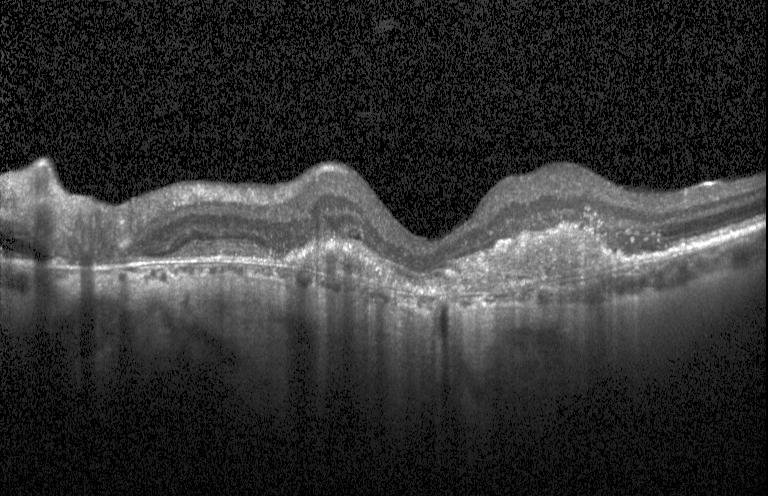
Macular OCT demonstrating a choroidal neovascular membrane.